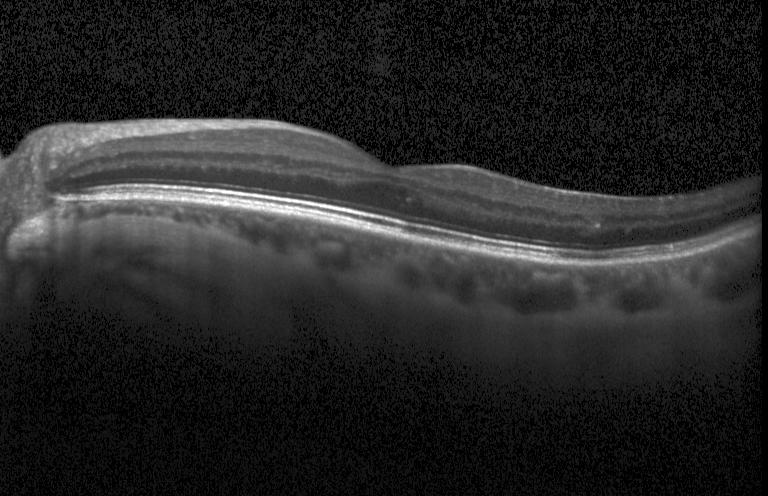

Centered on the fovea, retinal OCT cross-section.
Diagnosis: neither choroidal neovascularization, diabetic macular edema, nor drusen.